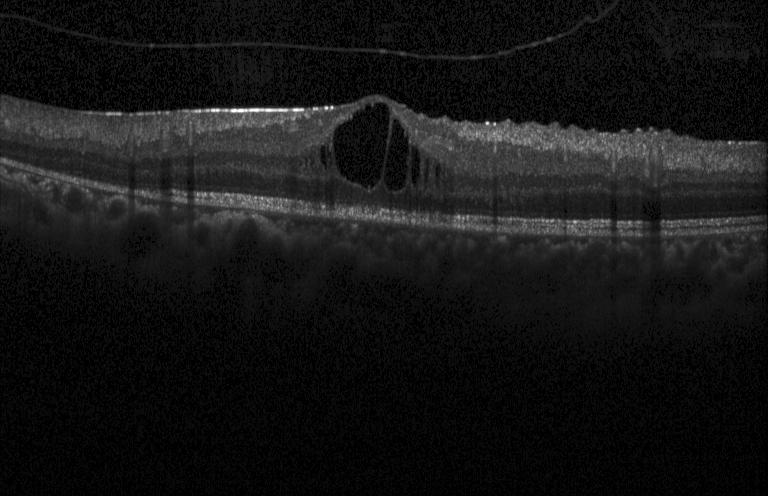
Instrument: Heidelberg Spectralis; optical coherence tomography scan
Diagnosis: DME.